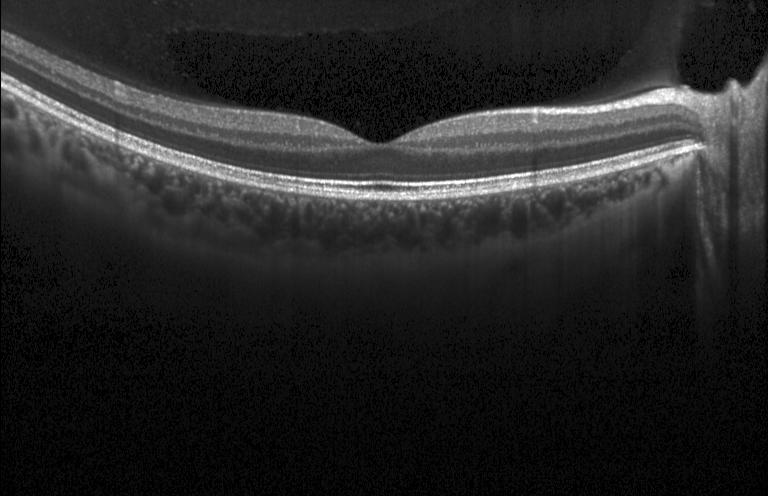 Spectral-domain OCT. OCT line scan. Dx: neither choroidal neovascularization, diabetic macular edema, nor drusen.